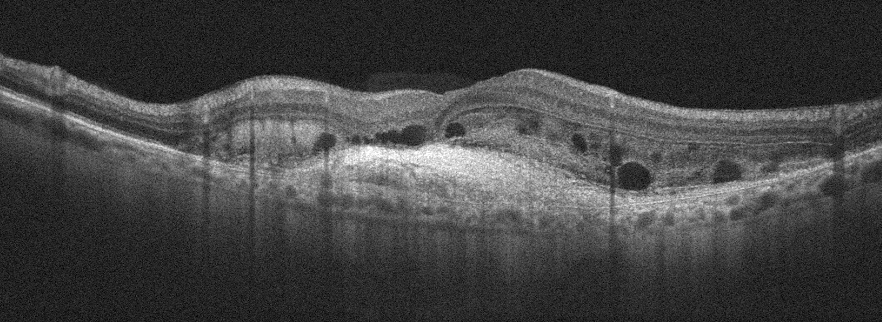

OCT B-scan showing age-related macular degeneration.